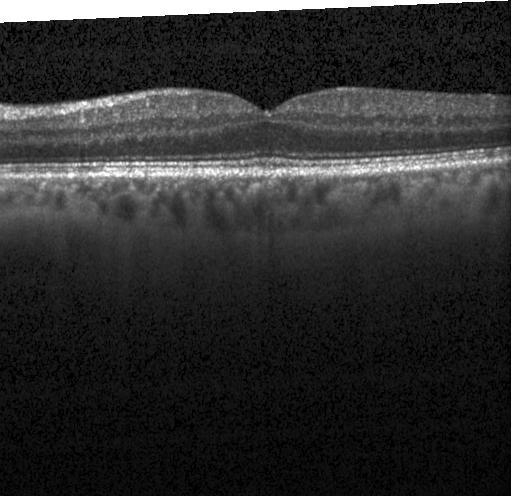
Optical coherence tomography scan — Macular OCT: no evidence of CNV, DME, or drusen.